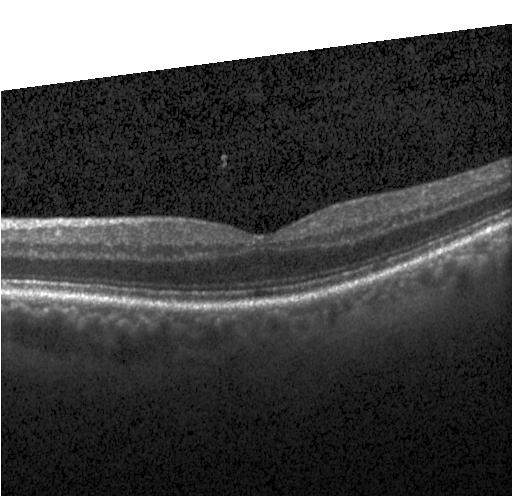
Macular scan · OCT B-scan · SD-OCT
Finding: no choroidal neovascularization, diabetic macular edema, or drusen.